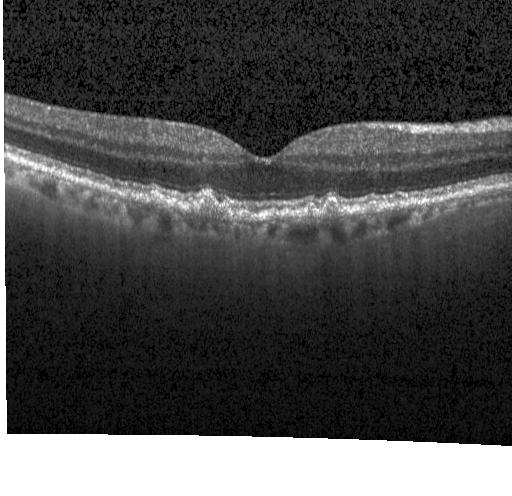

Finding: sub-RPE drusenoid deposits.